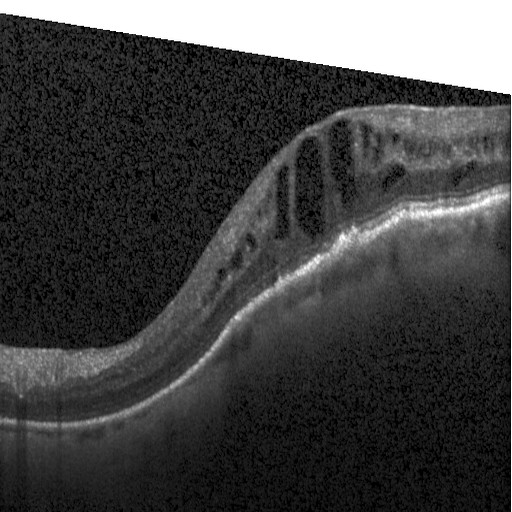

OCT B-scan, spectral-domain OCT
The scan shows DME.